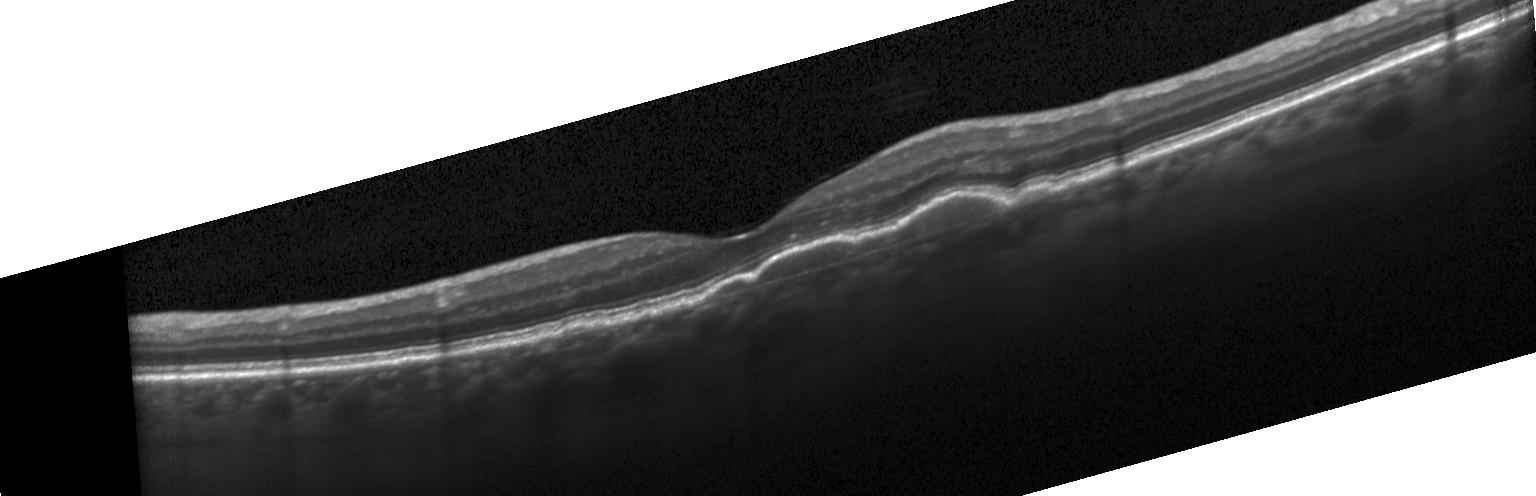 Assessment: a choroidal neovascular membrane.